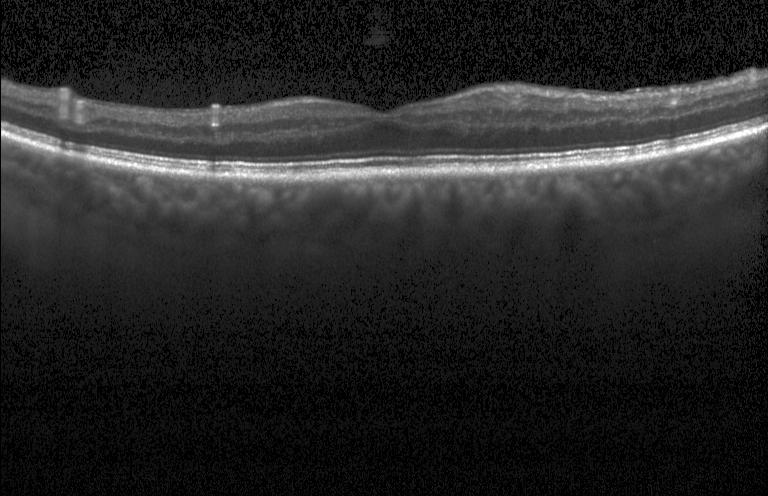
Diagnosis: neither CNV, DME, nor drusen.